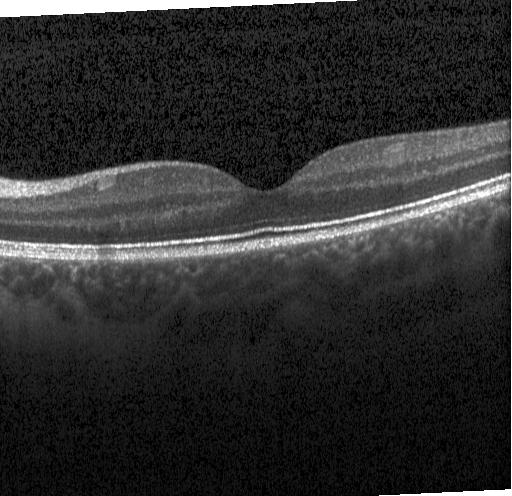 No CNV, no DME, and no drusen.